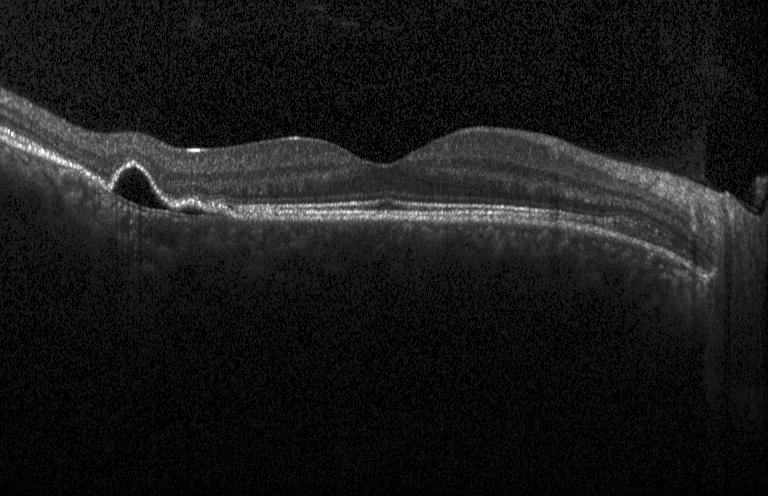
Retinal OCT B-scan — Impression: a choroidal neovascular membrane.